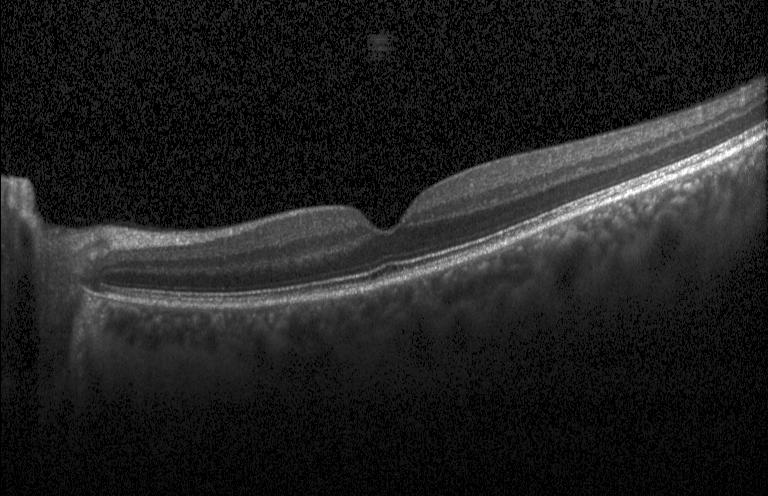

Impression: no choroidal neovascularization, no diabetic macular edema, and no drusen.